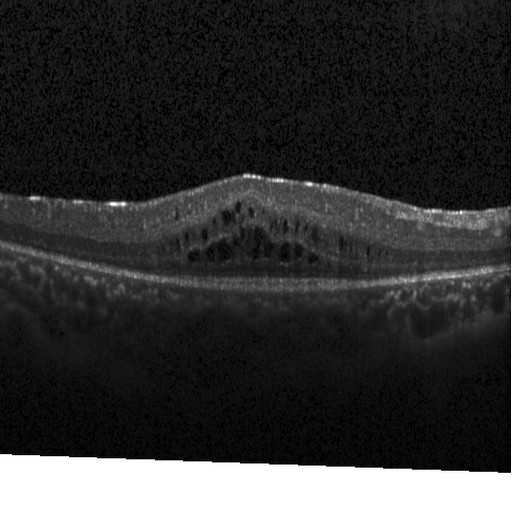
Retinal OCT B-scan; fovea-centered — Impression: diabetic macular edema (DME).